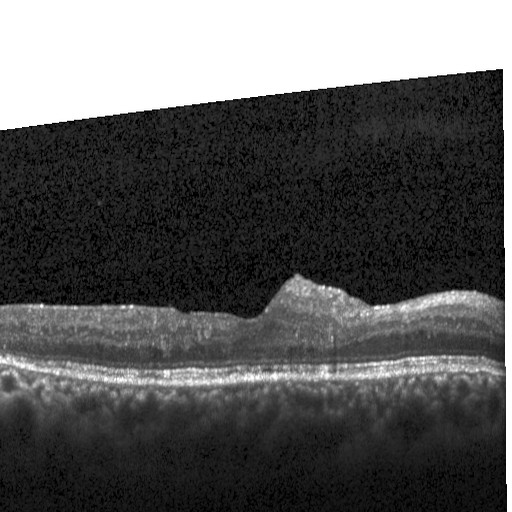
Fovea-centered · OCT line scan · SD-OCT.
This B-scan demonstrates DME.